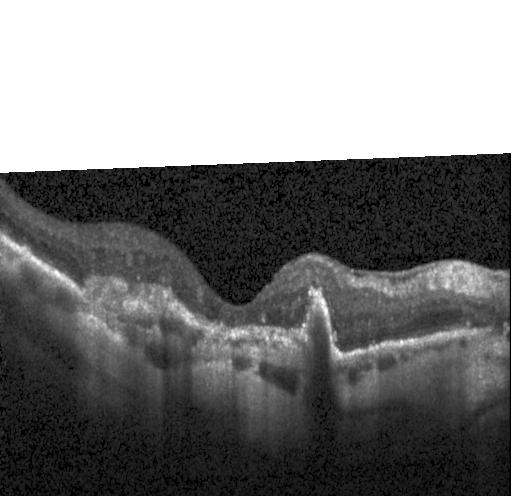

Optical coherence tomography scan
Impression: a choroidal neovascular membrane.